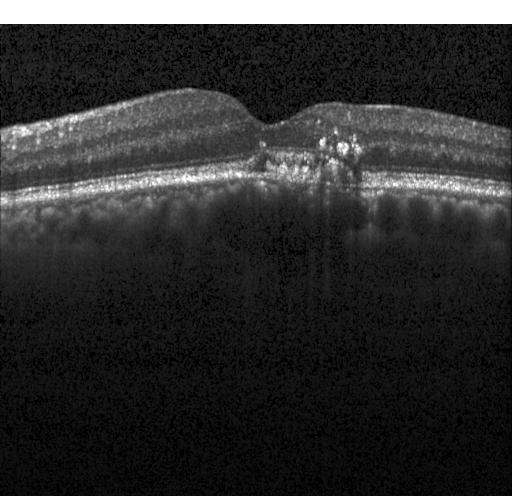

Fovea-centered · OCT line scan · acquired on a Heidelberg Spectralis · spectral-domain optical coherence tomography. Impression: CNV.